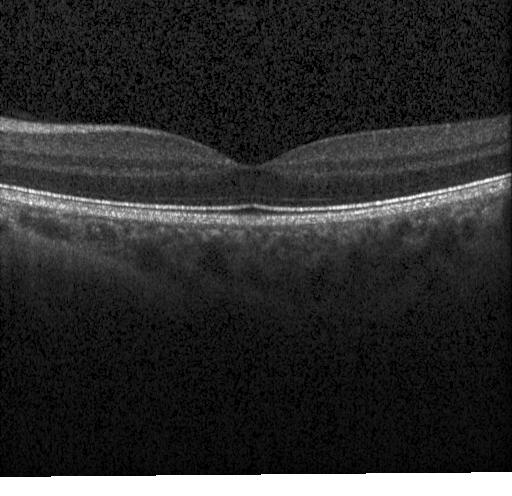

Spectral-domain OCT · optical coherence tomography scan
Impression: no choroidal neovascularization, diabetic macular edema, or drusen.